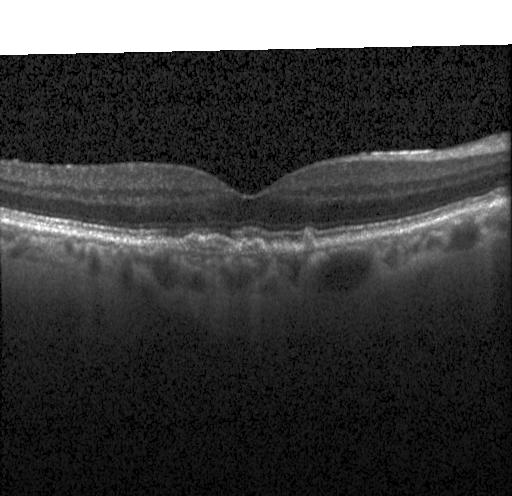

Optical coherence tomography B-scan
Dx: multiple drusen.